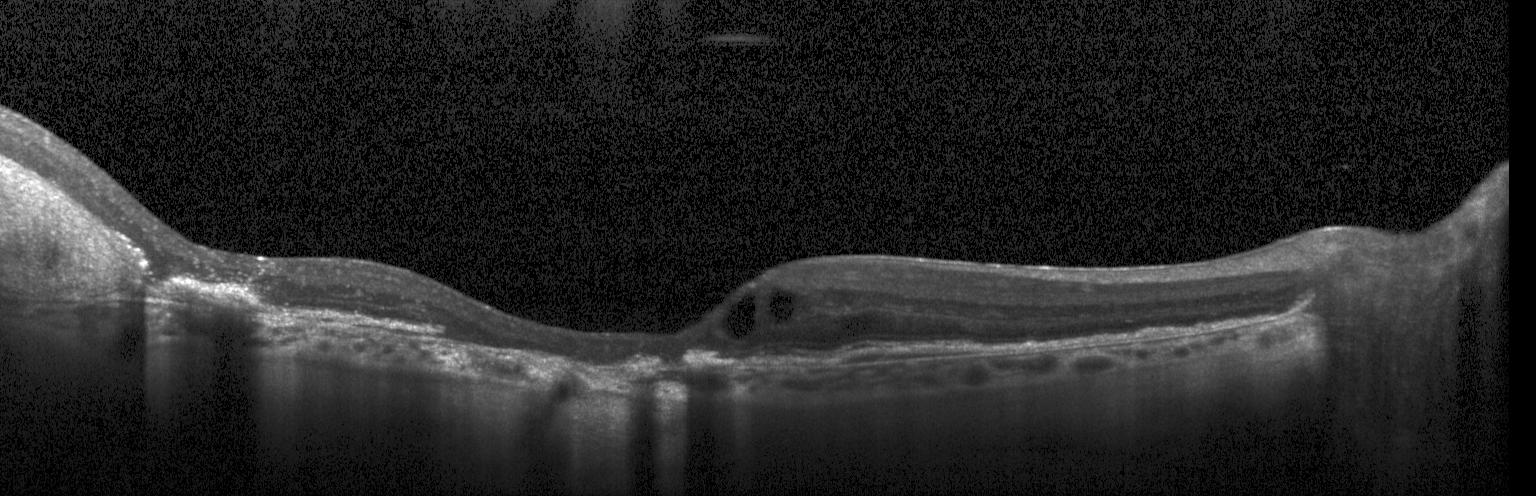
Heidelberg Spectralis; centered on the fovea; OCT B-scan — The scan shows a choroidal neovascular membrane.